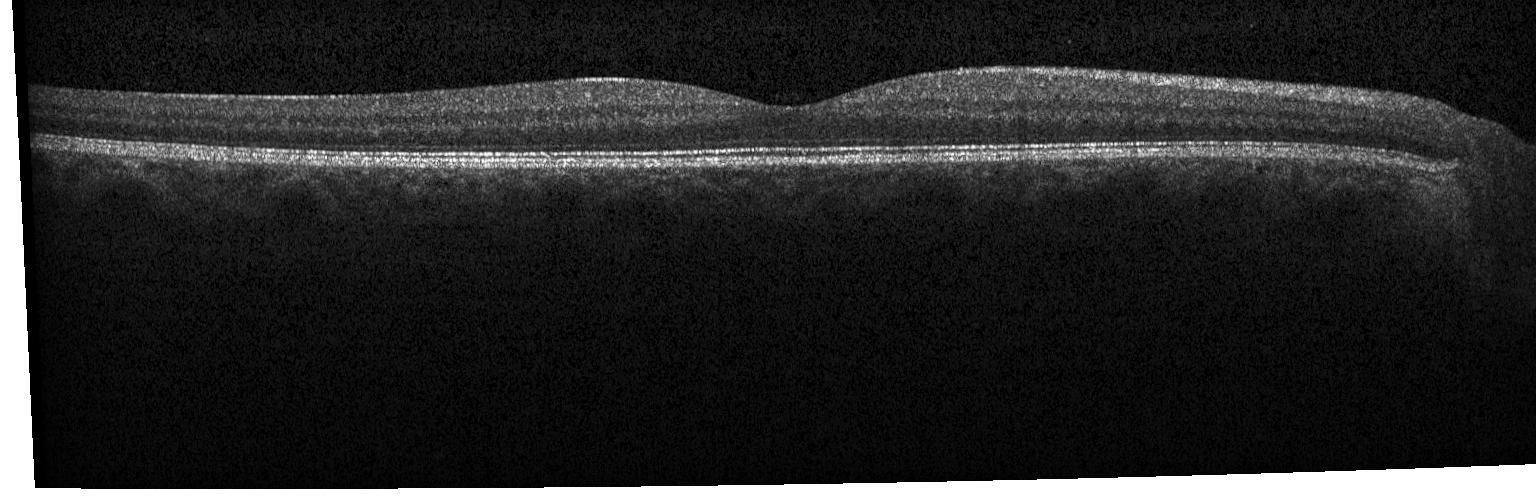
Instrument: Heidelberg Spectralis; retinal OCT B-scan; spectral-domain optical coherence tomography; macular scan.
Diagnosis: no CNV, DME, or drusen.